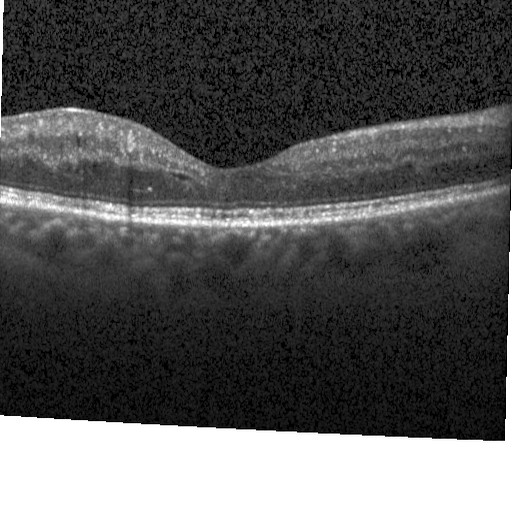

Optical coherence tomography scan. OCT finding: DME.